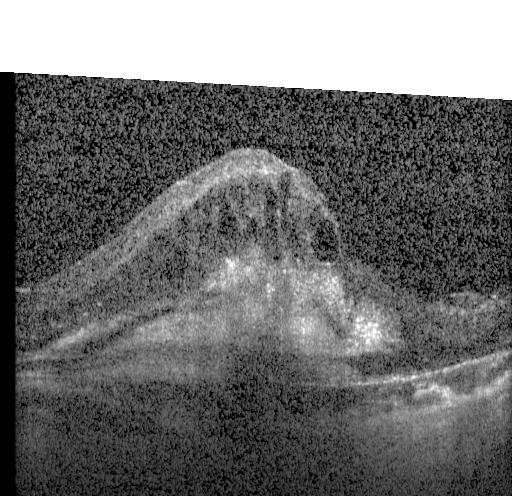 Finding: choroidal neovascularization (CNV).